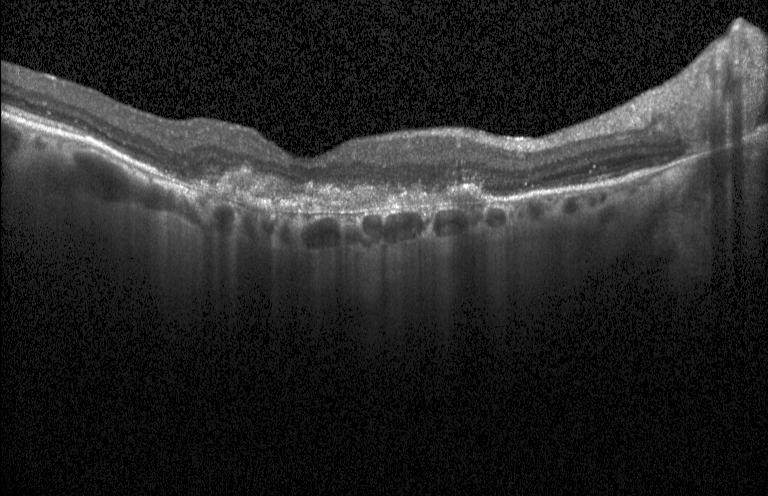 A choroidal neovascular membrane.